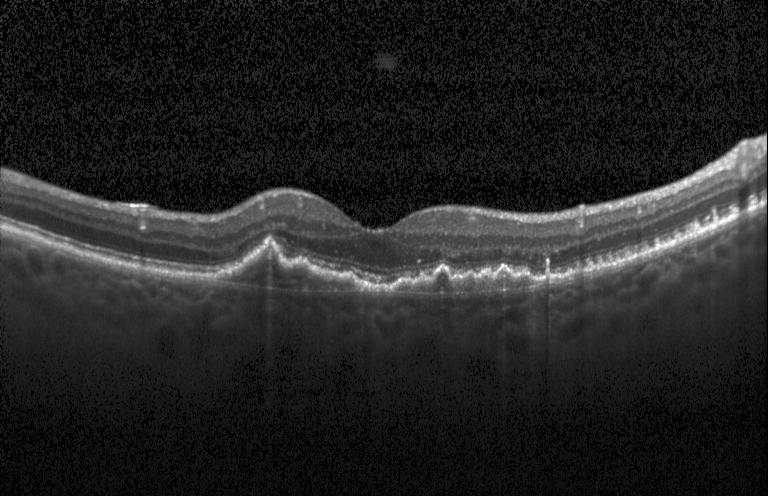
Dx: CNV.